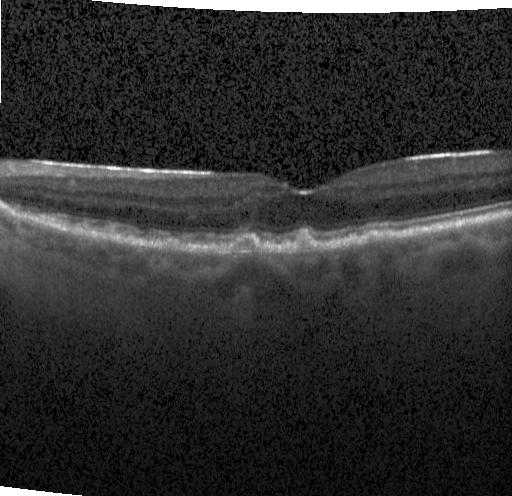

OCT scan showing multiple drusen.